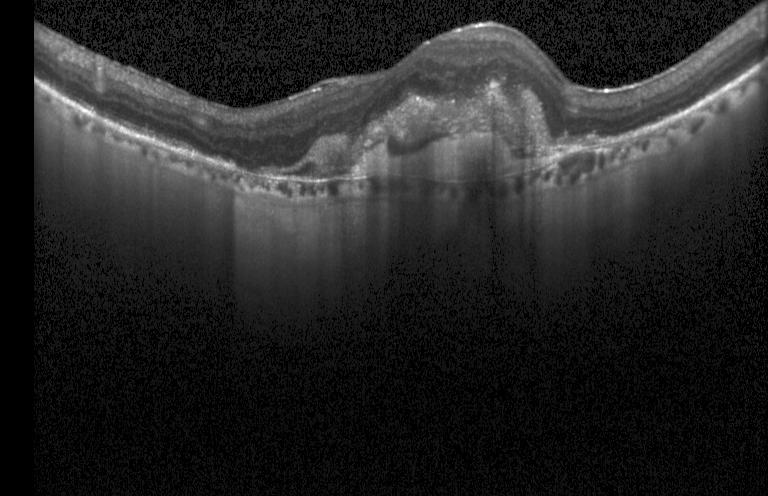
Heidelberg Spectralis OCT system, through the macula, SD-OCT, OCT B-scan — Diagnosis: a choroidal neovascular membrane.